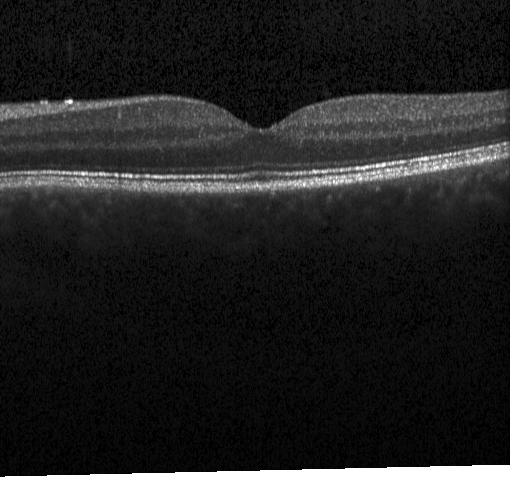 Diagnosis: neither choroidal neovascularization, diabetic macular edema, nor drusen.